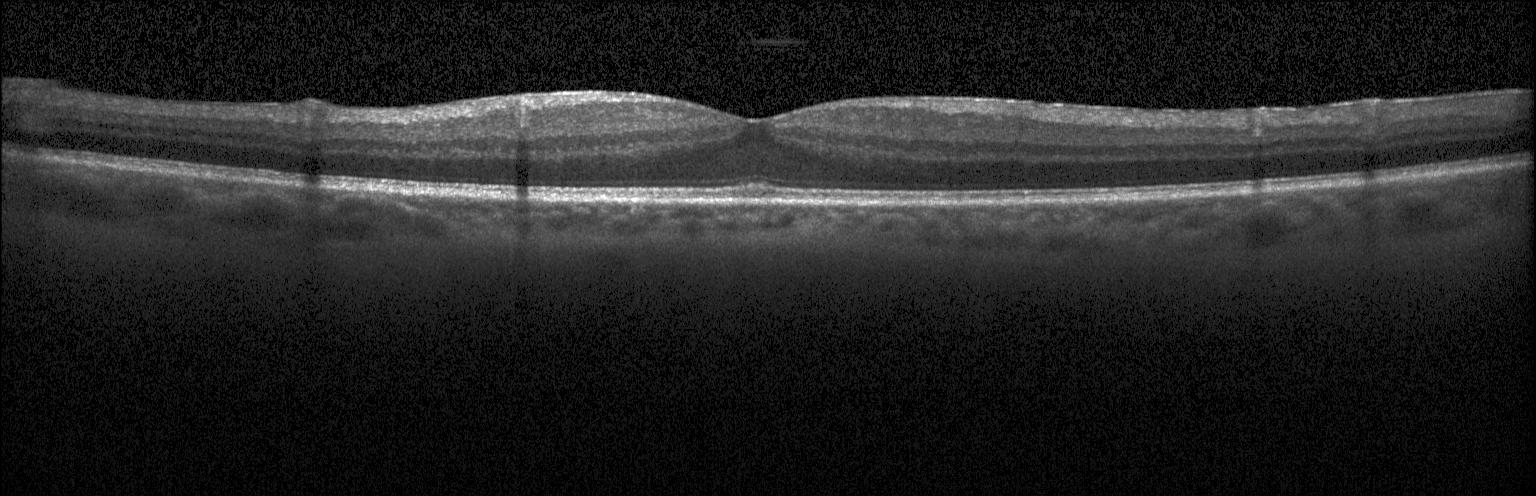 Impression: neither CNV, DME, nor drusen.